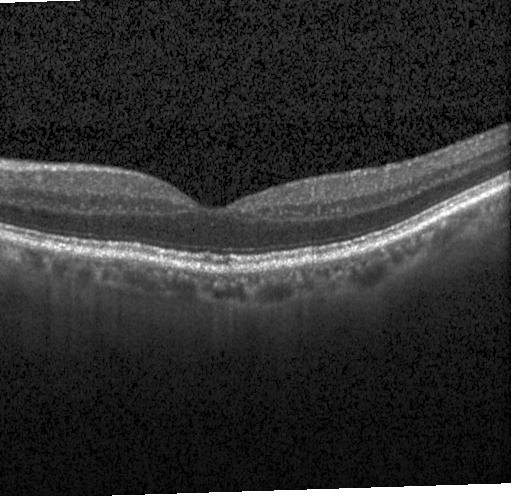

OCT line scan.
Diagnosis: no CNV, DME, or drusen.